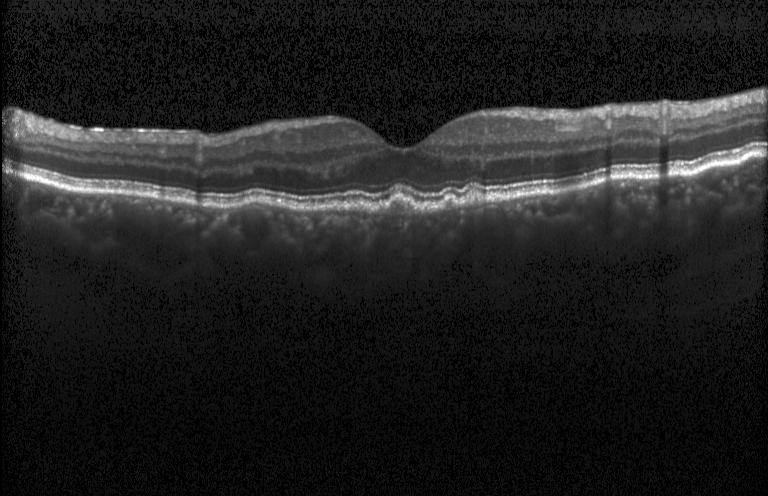 OCT line scan
Assessment: multiple drusen.